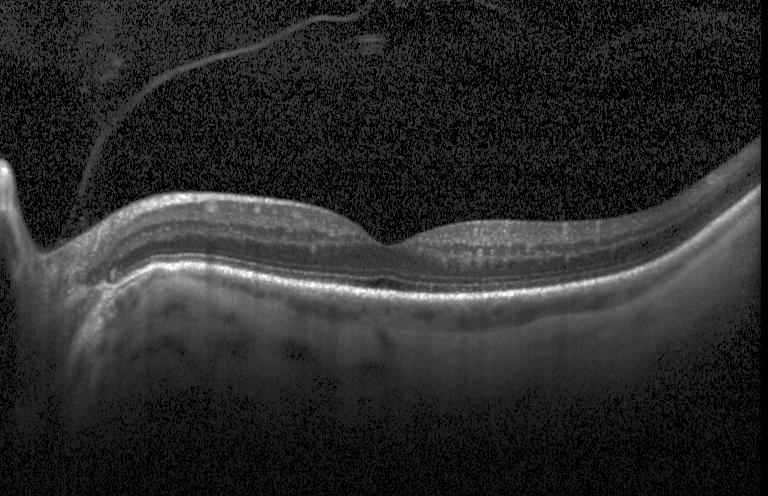 Optical coherence tomography B-scan. Impression: no evidence of choroidal neovascularization, diabetic macular edema, or drusen.